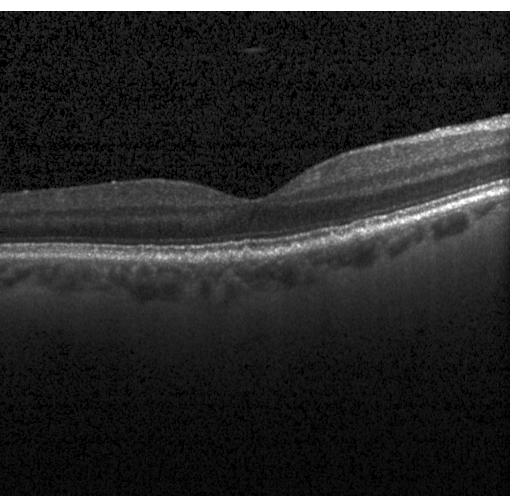
Spectral-domain optical coherence tomography, Heidelberg Spectralis OCT system, horizontal scan through the fovea, OCT B-scan
Sub-RPE drusenoid deposits.